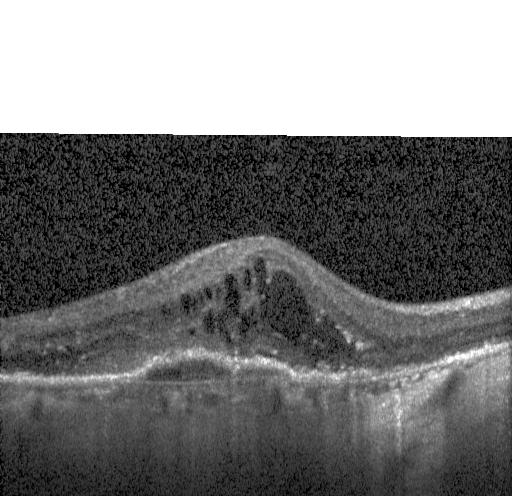 Retinal OCT cross-section; fovea-centered; Heidelberg Spectralis OCT system — Finding: choroidal neovascularization.